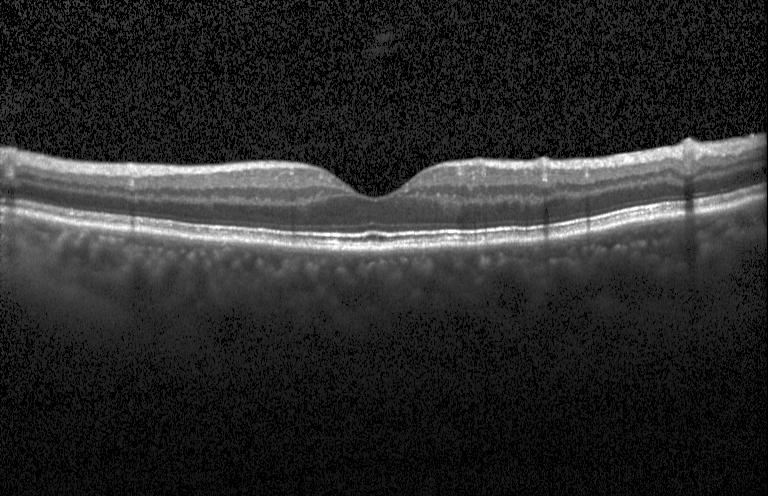 Optical coherence tomography B-scan. Finding: neither choroidal neovascularization, diabetic macular edema, nor drusen.